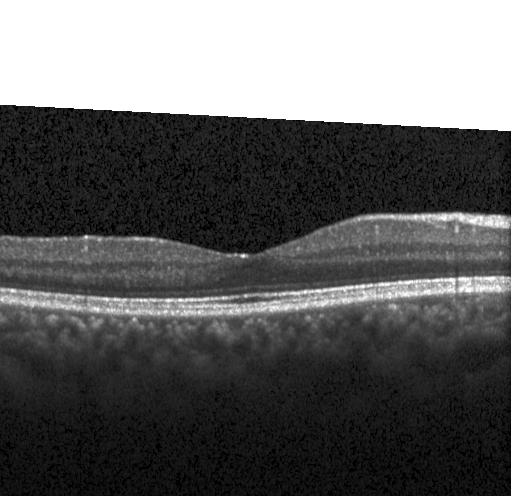
Instrument: Heidelberg Spectralis · OCT line scan · SD-OCT. This B-scan demonstrates no choroidal neovascularization, diabetic macular edema, or drusen.